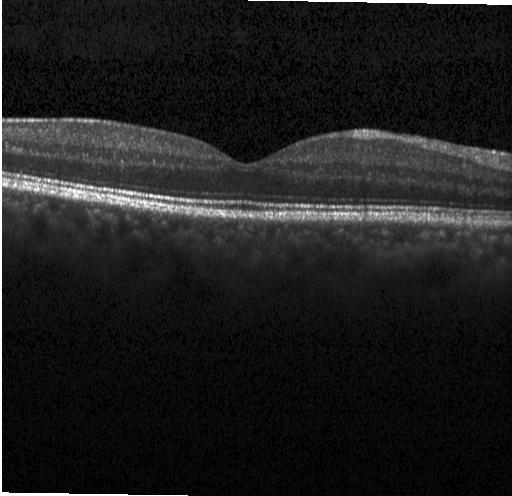

Heidelberg Spectralis OCT system; SD-OCT; OCT line scan
No choroidal neovascularization, no diabetic macular edema, and no drusen.